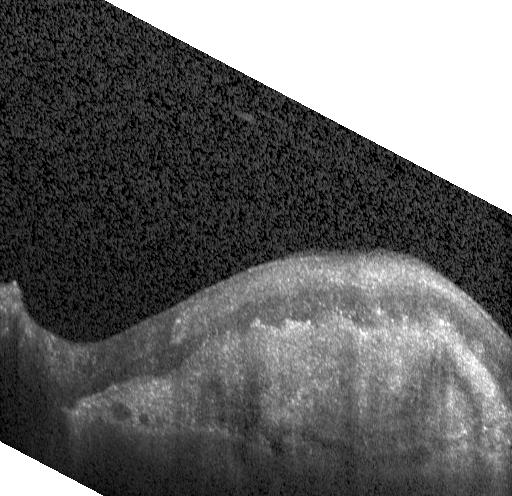 Dx: choroidal neovascularization (CNV).